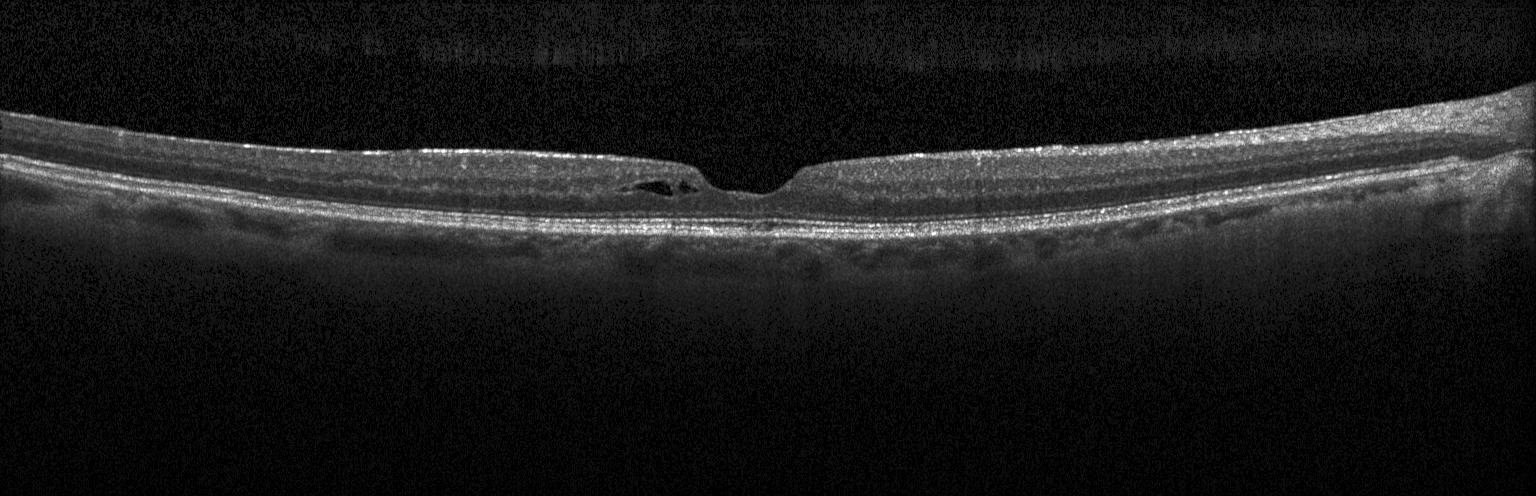
OCT line scan; fovea-centered.
Impression: DME.